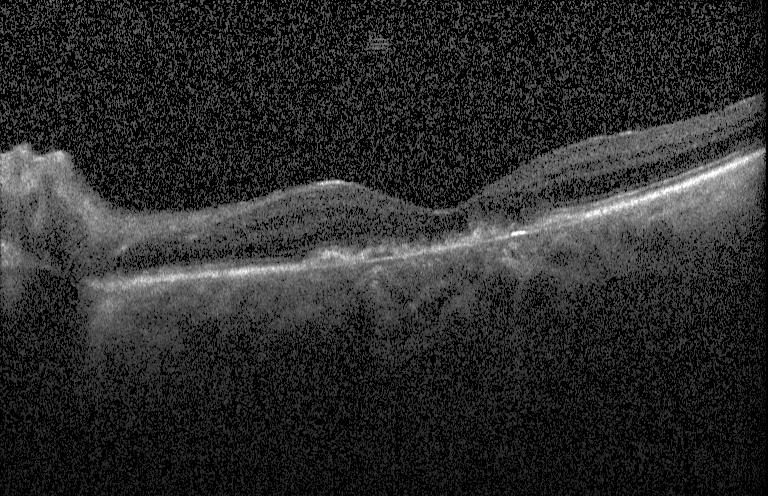 Finding: CNV.